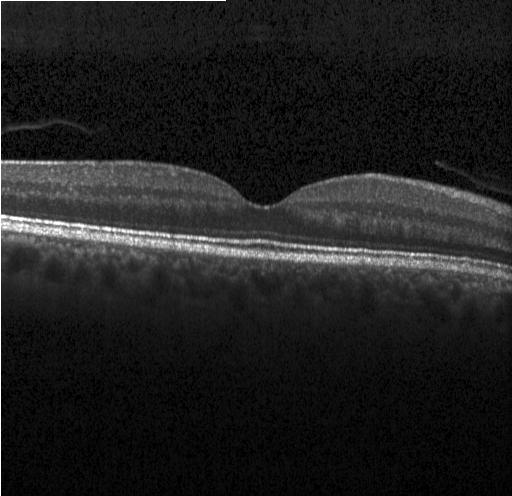

Through the macula; OCT line scan; acquired on a Heidelberg Spectralis
Diagnosis: no evidence of CNV, DME, or drusen.